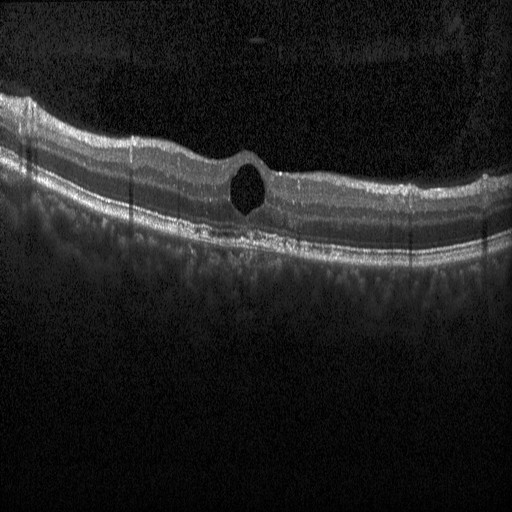

DME.